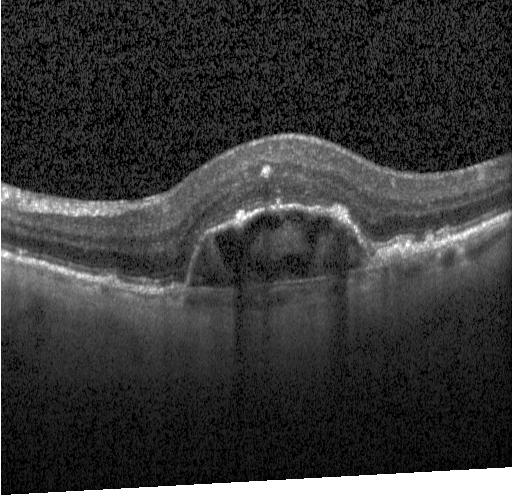

OCT line scan. The scan shows choroidal neovascularization (CNV).